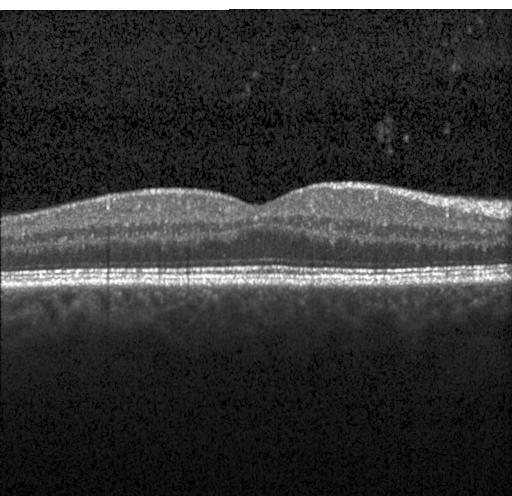 Centered on the fovea. Heidelberg Spectralis. Optical coherence tomography B-scan. Spectral-domain optical coherence tomography — The scan shows no evidence of CNV, DME, or drusen.